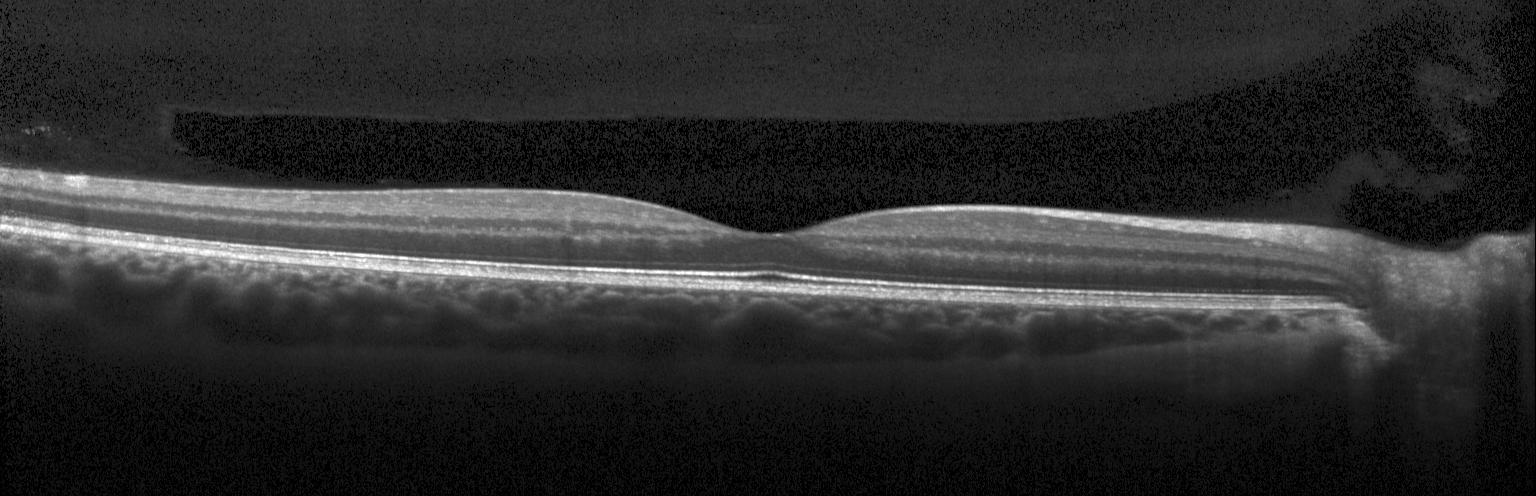

Impression: neither choroidal neovascularization, diabetic macular edema, nor drusen.